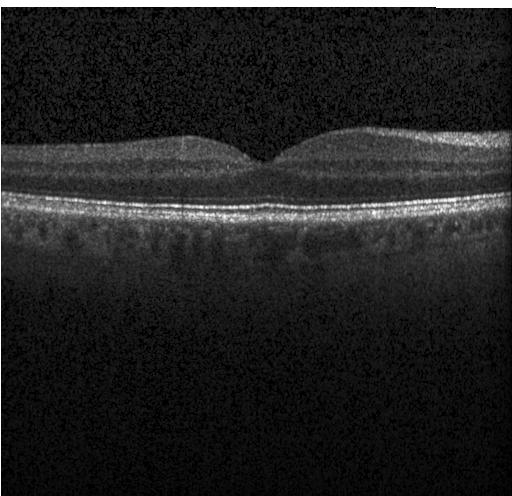
Retinal OCT cross-section
Impression: no evidence of choroidal neovascularization, diabetic macular edema, or drusen.